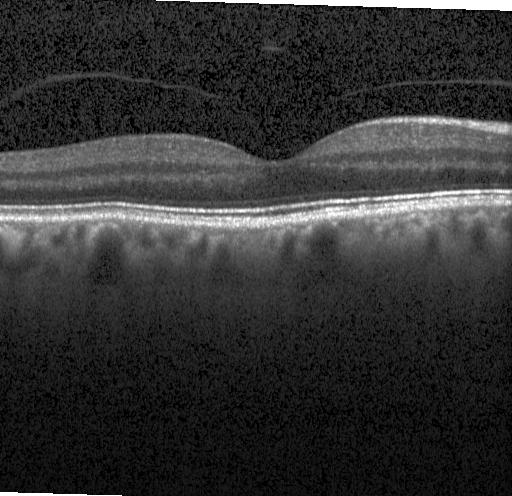
Optical coherence tomography scan — Impression: neither choroidal neovascularization, diabetic macular edema, nor drusen.